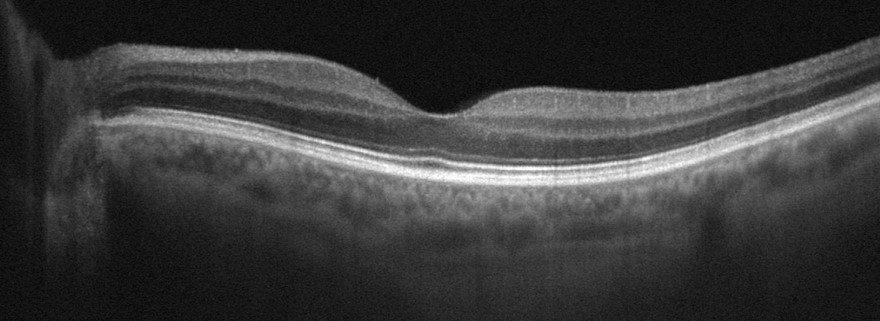

Fovea-centered · optical coherence tomography B-scan
Finding: no AMD, DME, ERM, RAO, RVO, or VID.